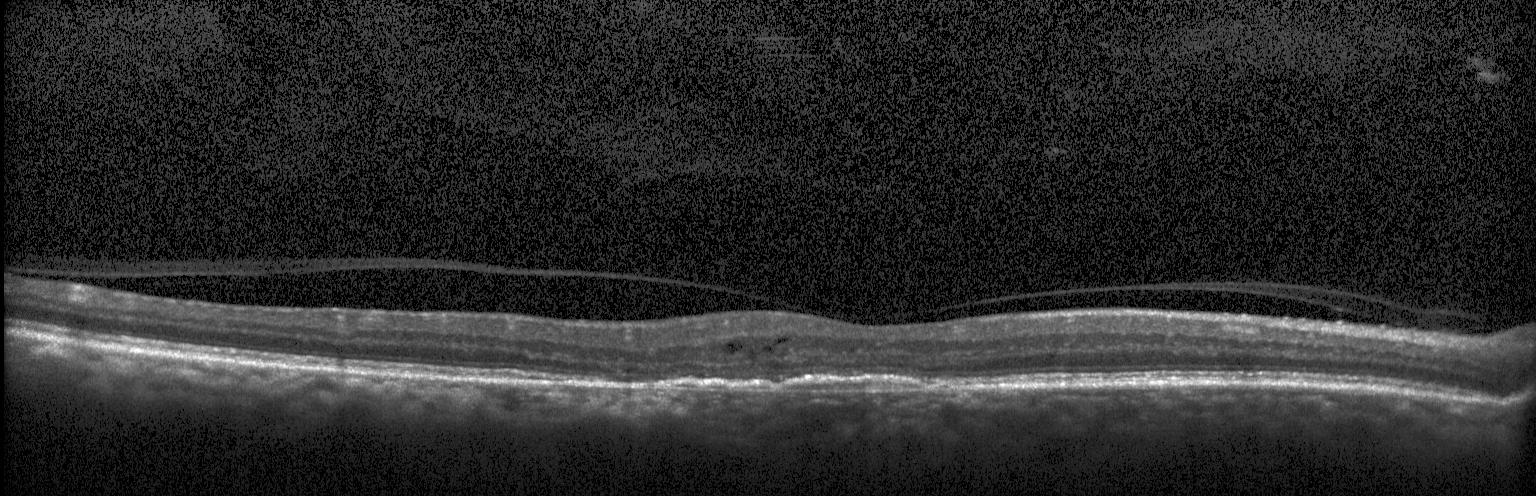 Spectral-domain optical coherence tomography; retinal OCT cross-section; centered on the fovea.
OCT finding: a choroidal neovascular membrane.